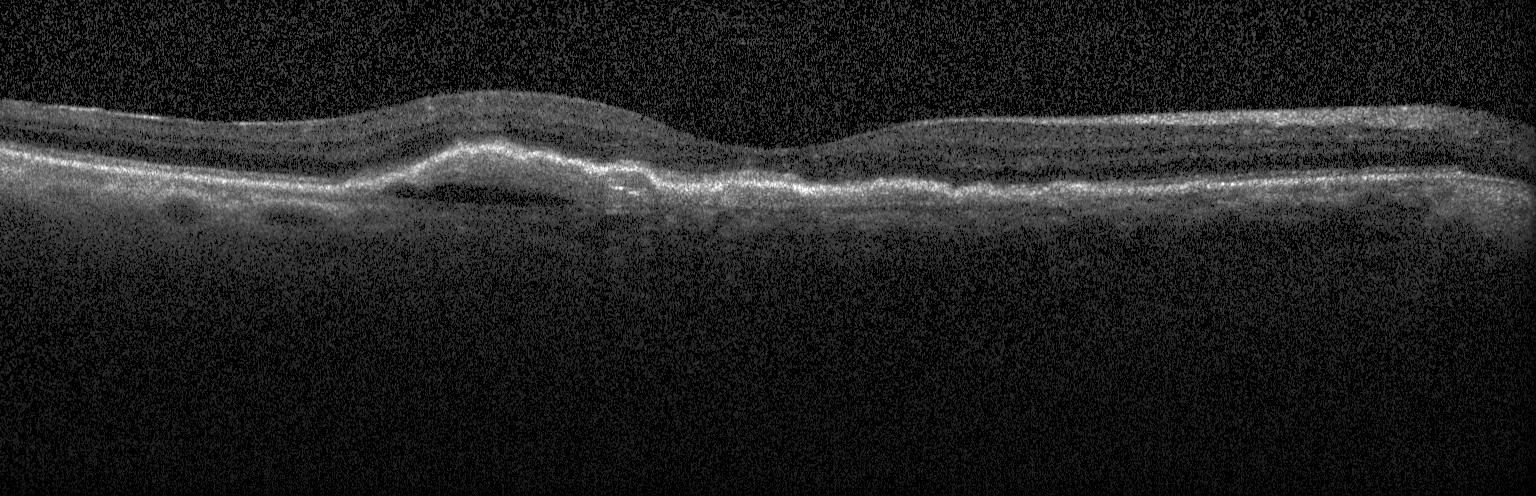
SD-OCT; OCT B-scan.
Diagnosis: choroidal neovascularization.